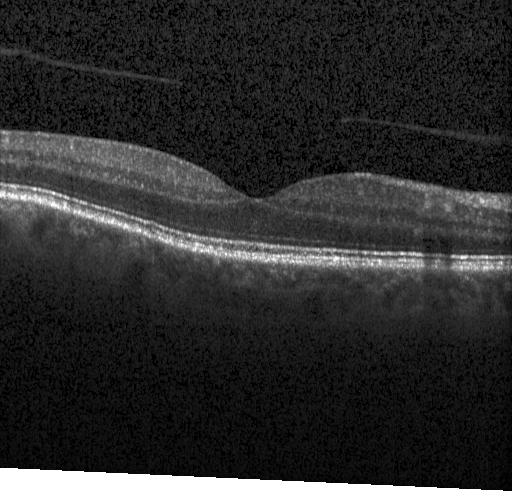 Centered on the fovea. Instrument: Heidelberg Spectralis. Retinal OCT cross-section
Assessment: no choroidal neovascularization, diabetic macular edema, or drusen.